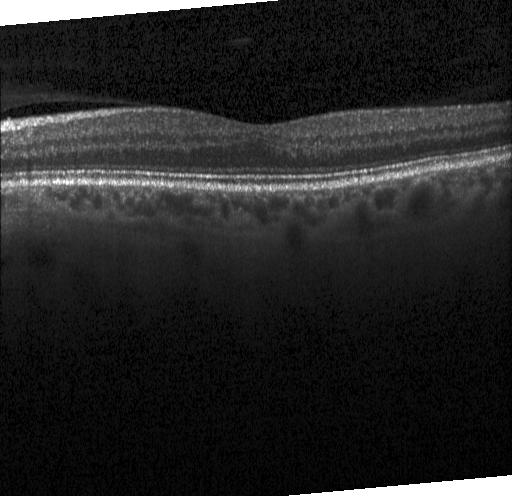

OCT B-scan showing no choroidal neovascularization, diabetic macular edema, or drusen.